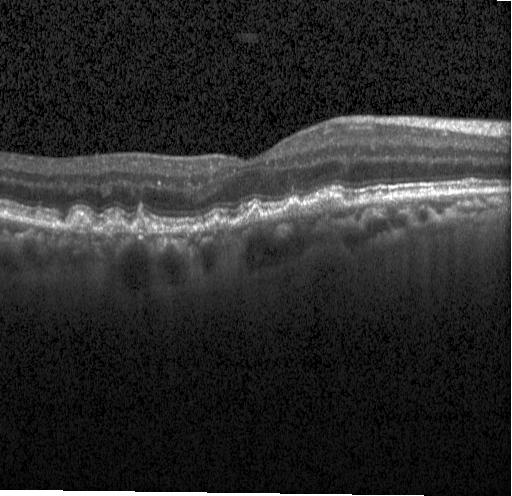 Retinal OCT B-scan.
This B-scan demonstrates drusen.